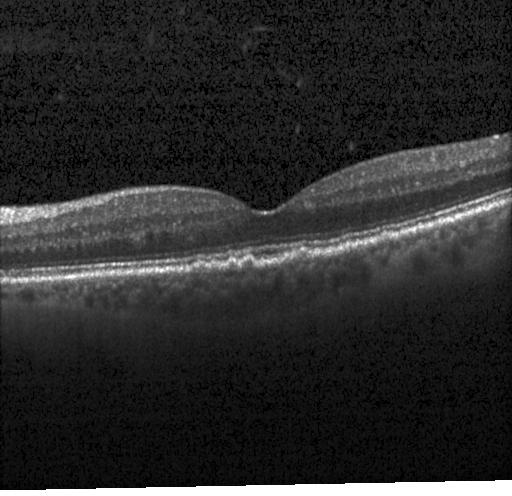

OCT B-scan, instrument: Heidelberg Spectralis, SD-OCT, fovea-centered
Drusen.